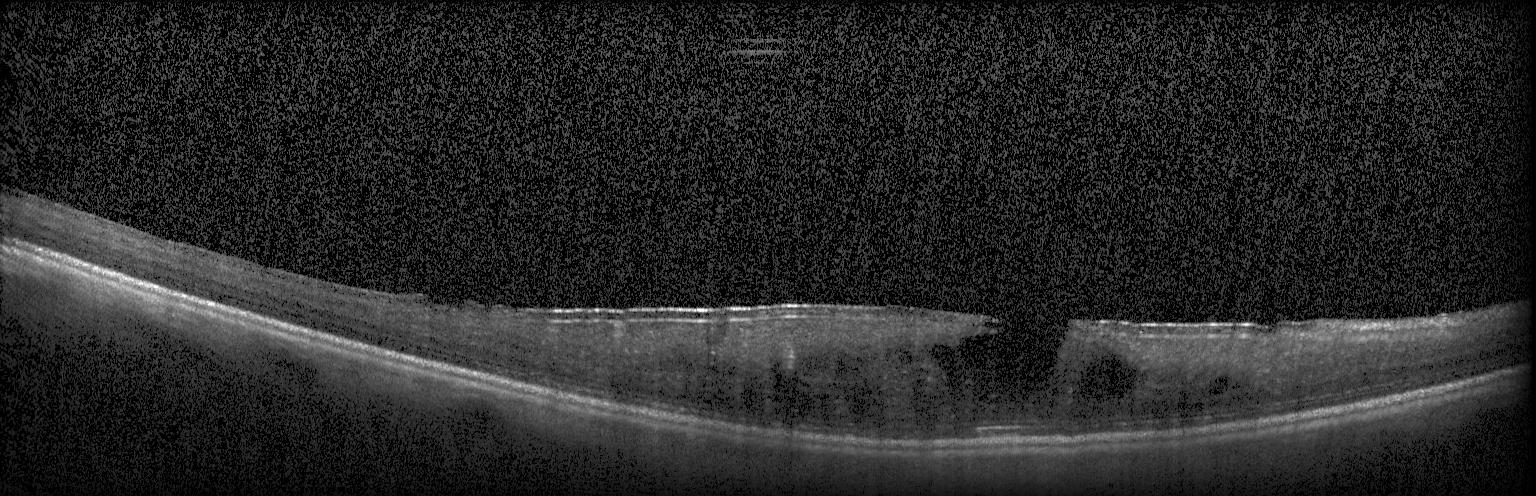
Acquired on a Heidelberg Spectralis, retinal OCT cross-section, SD-OCT — Diabetic macular edema.